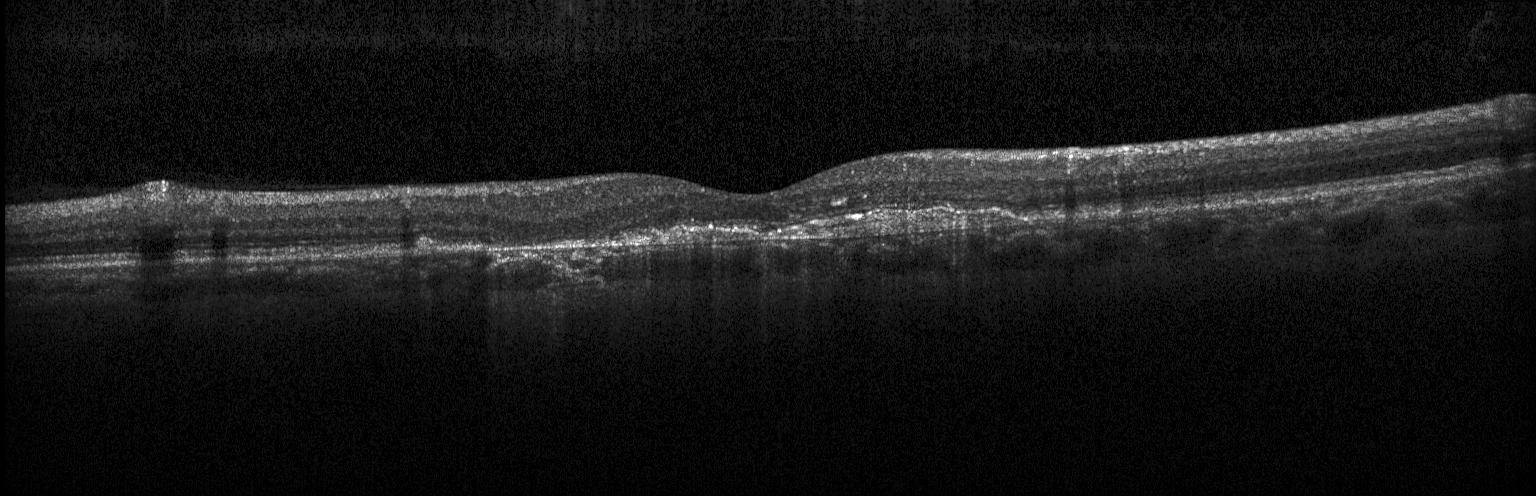
Macular OCT: no choroidal neovascularization, diabetic macular edema, or drusen.